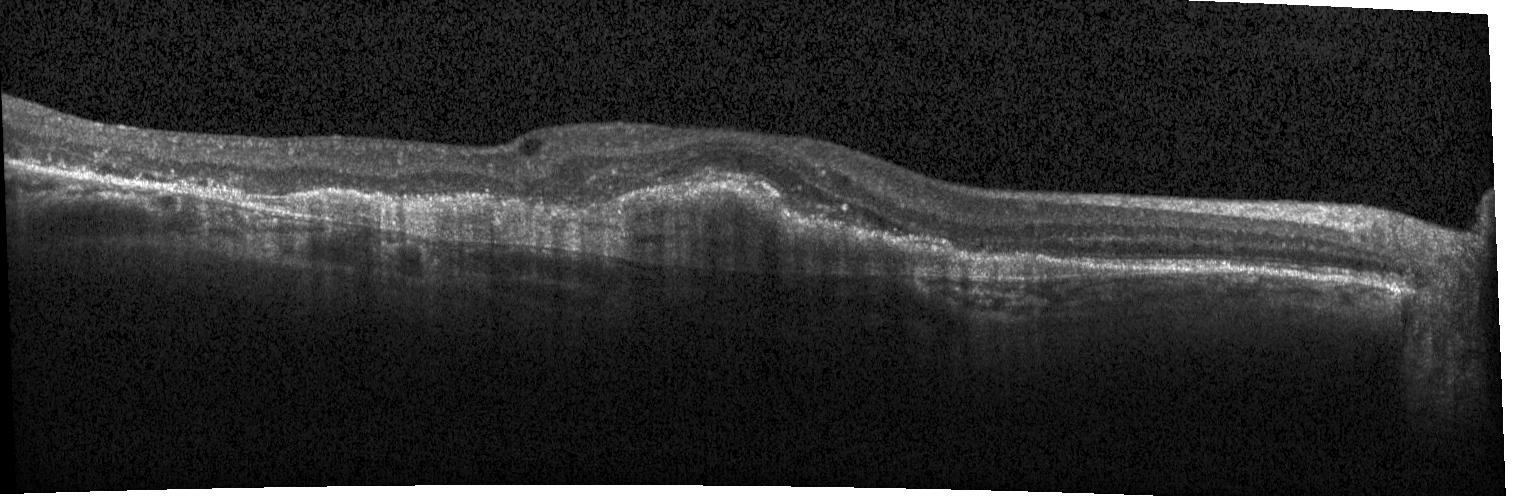 Acquired on a Heidelberg Spectralis; OCT B-scan — This B-scan demonstrates CNV.